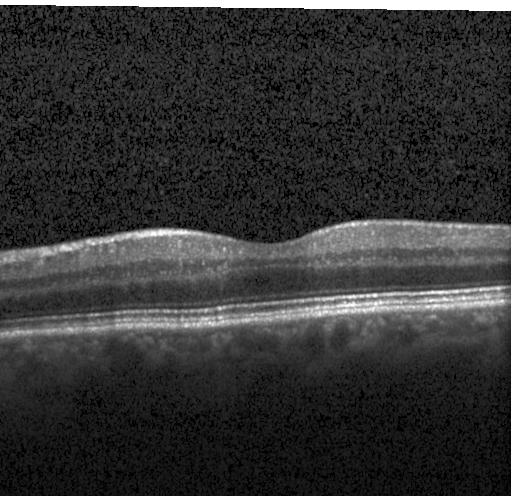 Dx: neither CNV, DME, nor drusen.